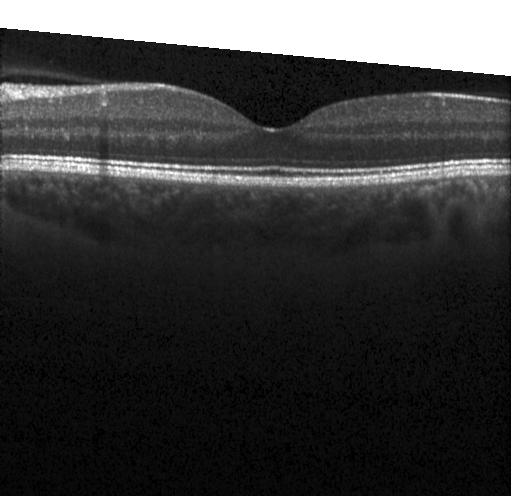

Retinal OCT B-scan — The scan shows no evidence of CNV, DME, or drusen.